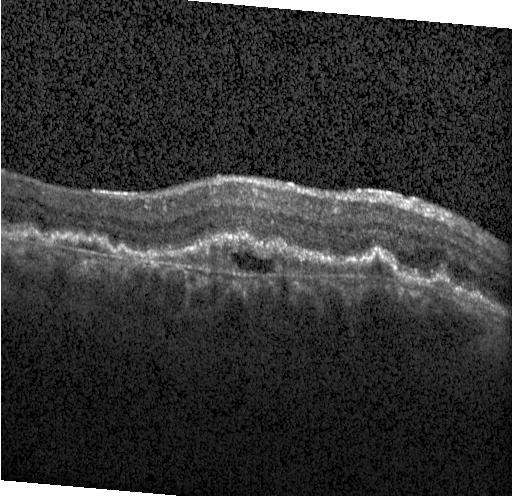 Macular OCT demonstrating choroidal neovascularization (CNV).